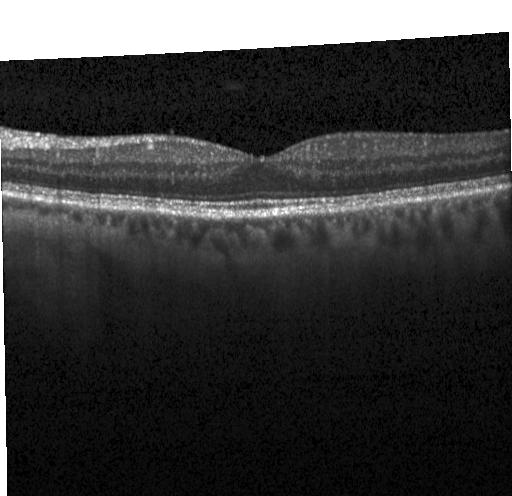 Acquired on a Heidelberg Spectralis, OCT line scan, spectral-domain OCT.
OCT finding: no choroidal neovascularization, diabetic macular edema, or drusen.